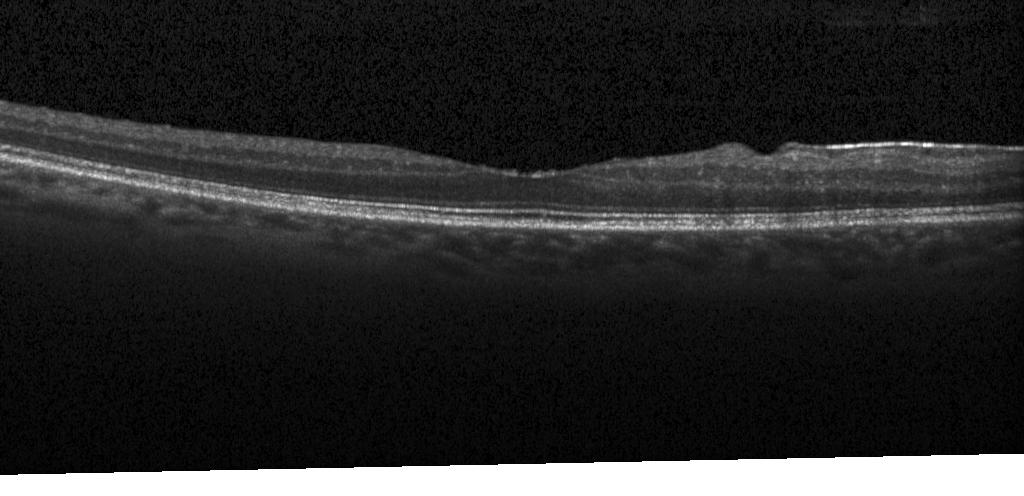

OCT finding: no CNV, DME, or drusen.